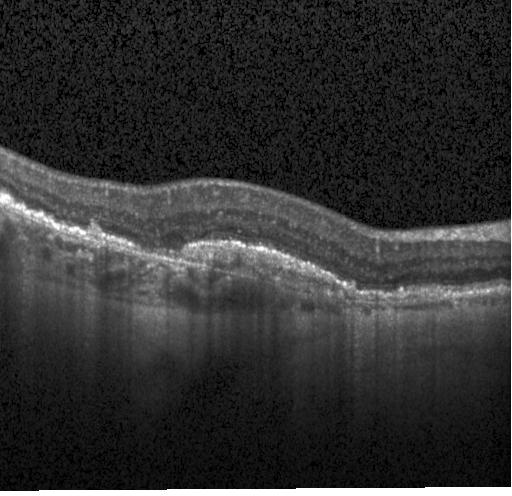
This B-scan demonstrates CNV.